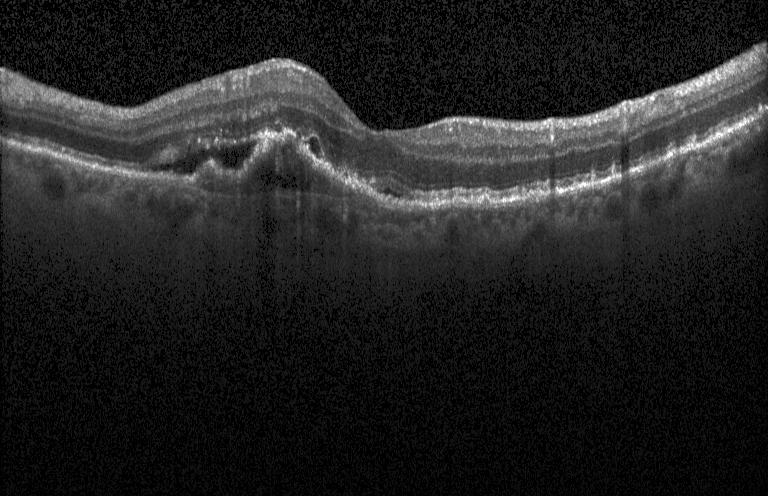 Impression: a choroidal neovascular membrane.